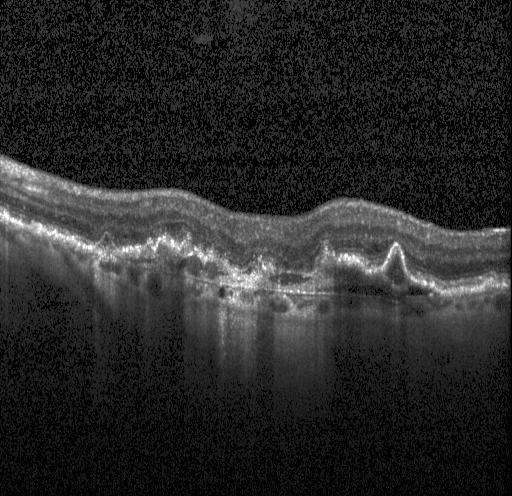 Horizontal scan through the fovea. OCT line scan. SD-OCT.
Finding: choroidal neovascularization (CNV).